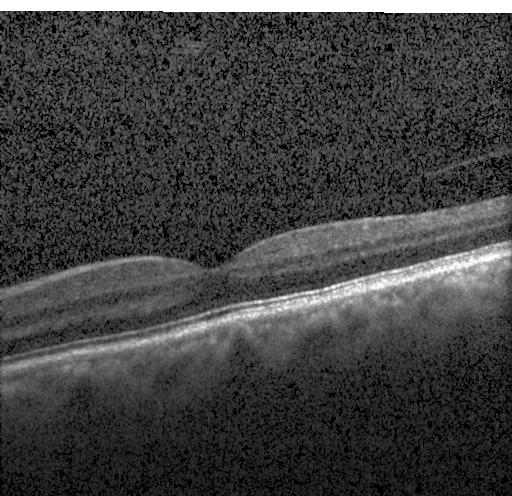

Diagnosis: neither choroidal neovascularization, diabetic macular edema, nor drusen.